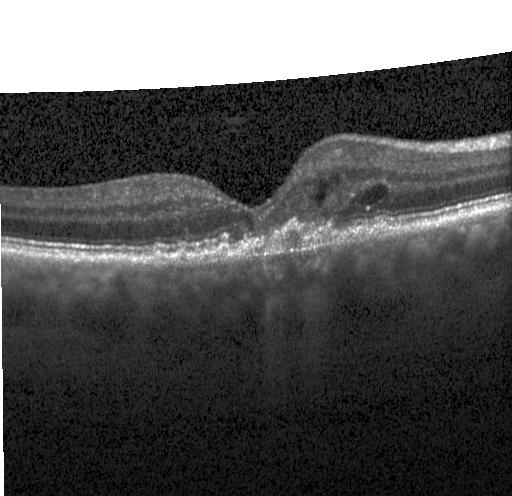

OCT line scan, spectral-domain optical coherence tomography. Finding: a choroidal neovascular membrane.